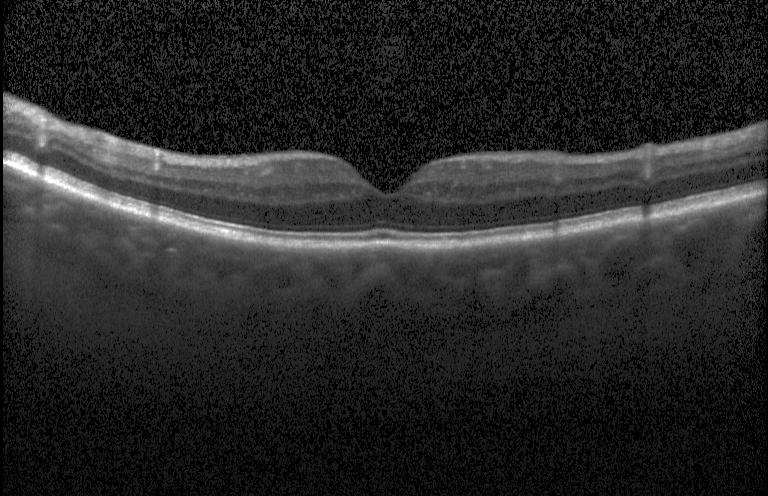
Neither choroidal neovascularization, diabetic macular edema, nor drusen.